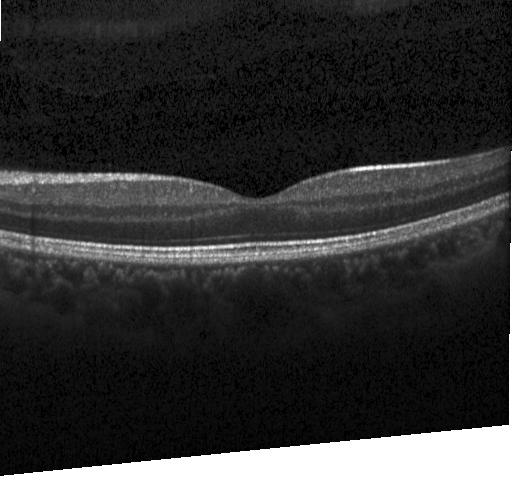
Finding: neither CNV, DME, nor drusen.